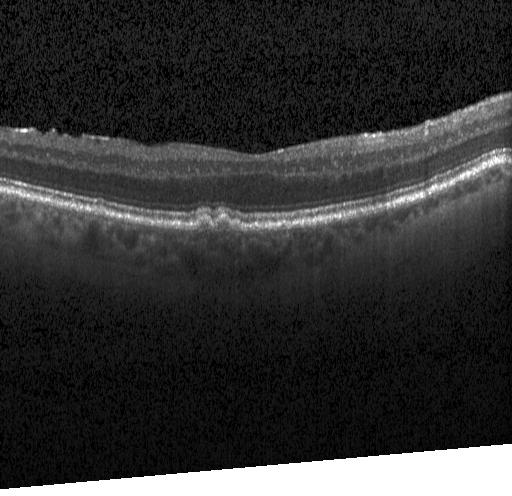 Macular scan · Heidelberg Spectralis OCT system · spectral-domain OCT · OCT B-scan.
This B-scan demonstrates sub-RPE drusenoid deposits.